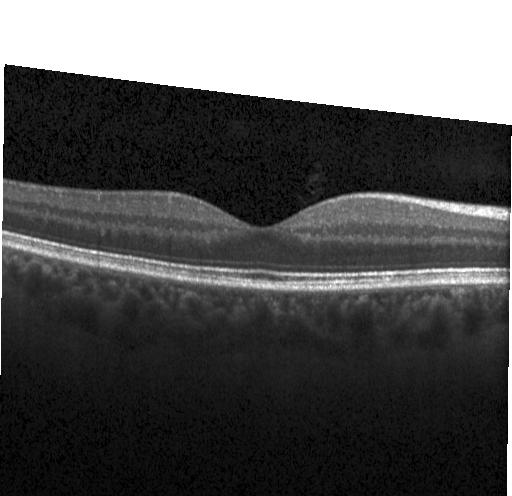
Optical coherence tomography B-scan · fovea-centered · acquired on a Heidelberg Spectralis. Assessment: neither CNV, DME, nor drusen.